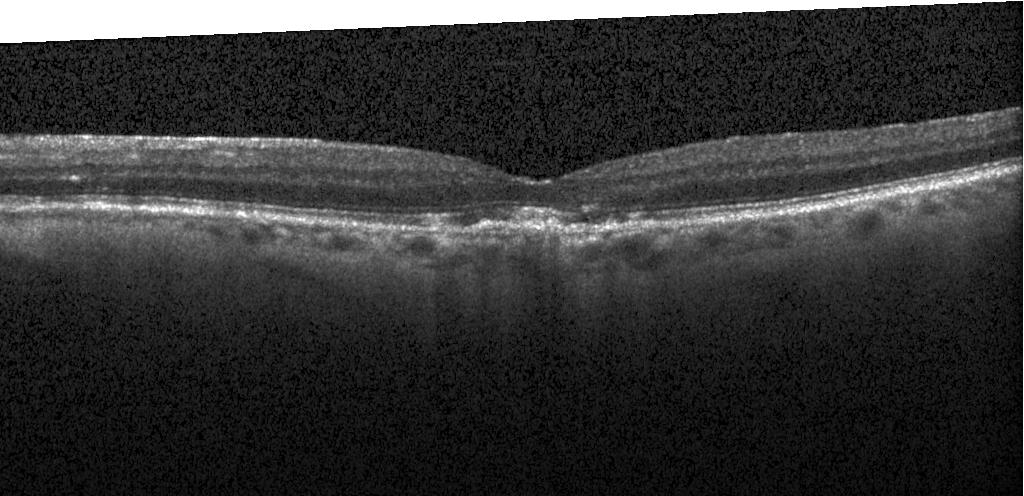

Assessment: CNV.